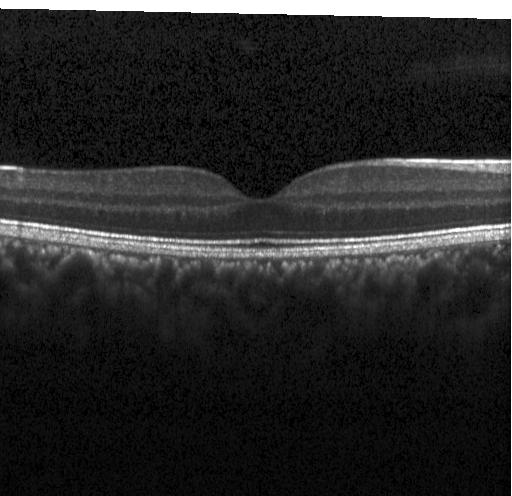
Impression: no choroidal neovascularization, diabetic macular edema, or drusen.